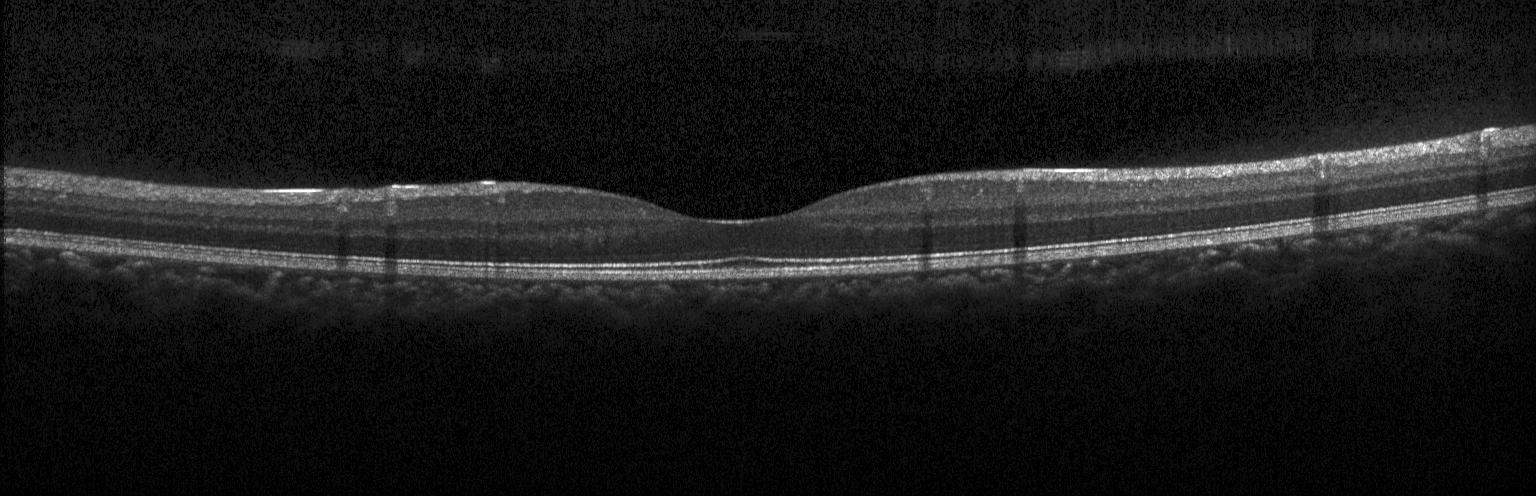

Retinal OCT cross-section — No choroidal neovascularization, no diabetic macular edema, and no drusen.